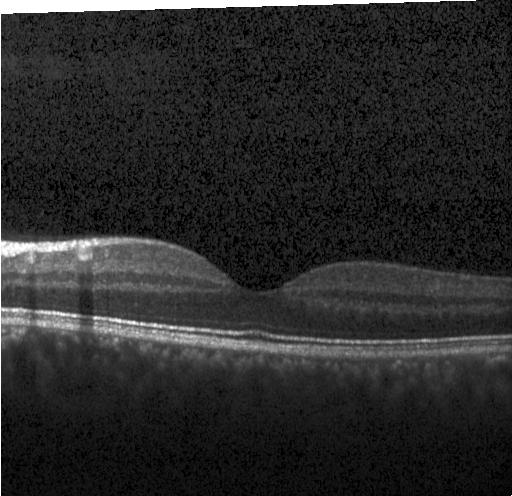

OCT line scan.
This B-scan demonstrates neither choroidal neovascularization, diabetic macular edema, nor drusen.